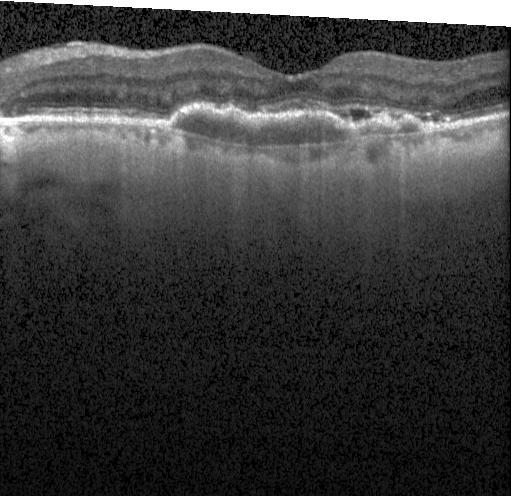

Finding: choroidal neovascularization.